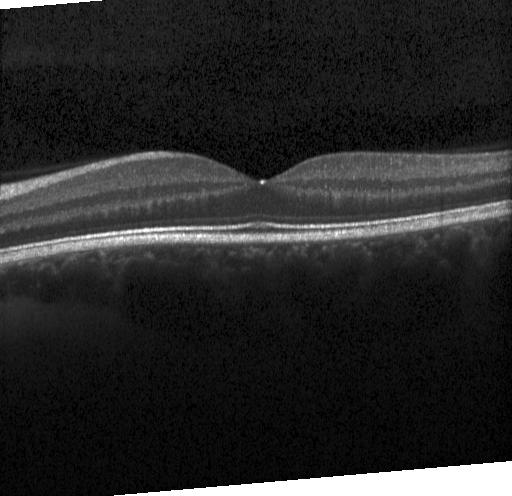
Retinal OCT B-scan. Spectral-domain OCT. Fovea-centered. Finding: no CNV, DME, or drusen.